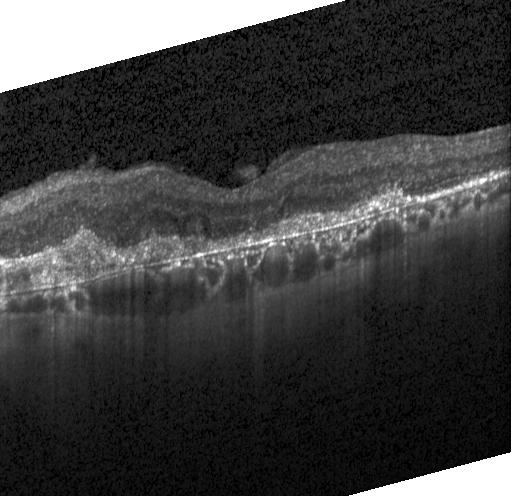 OCT line scan. Finding: a choroidal neovascular membrane.